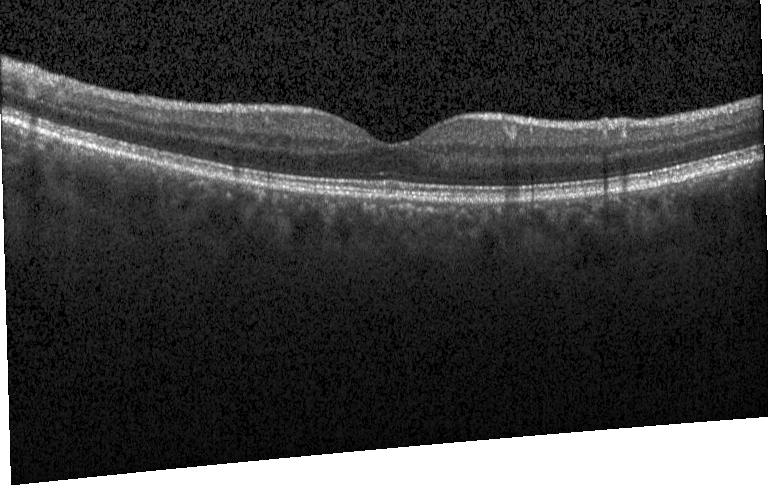 Retinal OCT cross-section.
This B-scan demonstrates no choroidal neovascularization, diabetic macular edema, or drusen.